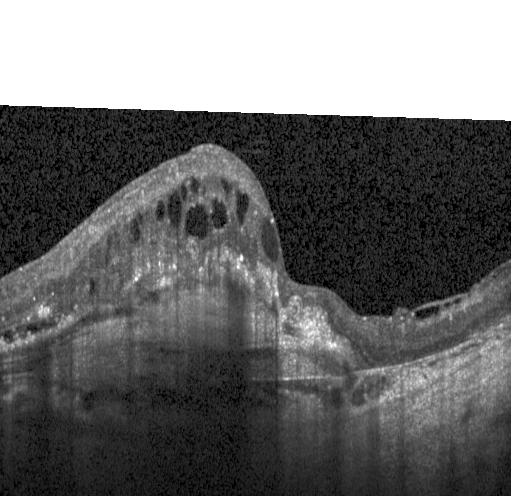

OCT line scan · Heidelberg Spectralis OCT system · spectral-domain OCT — The scan shows choroidal neovascularization (CNV).